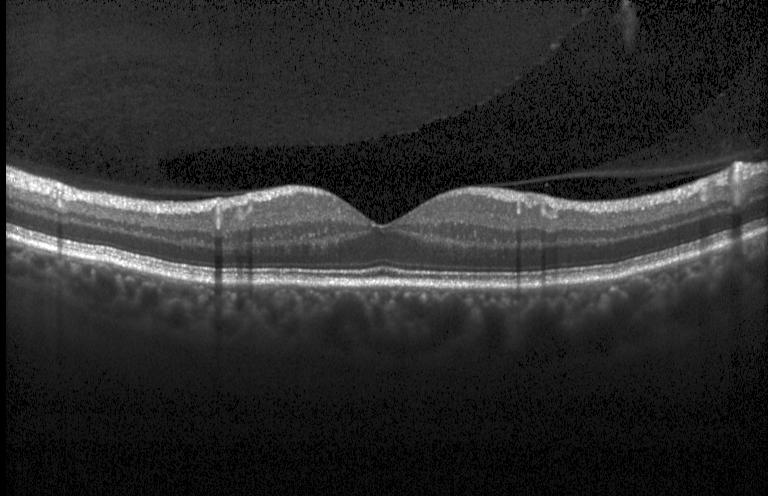
Retinal OCT cross-section — Macular OCT: no choroidal neovascularization, no diabetic macular edema, and no drusen.